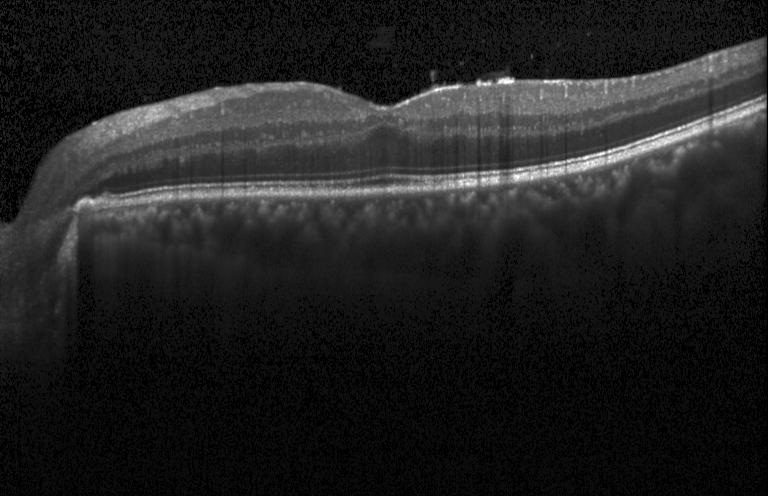 Fovea-centered, optical coherence tomography scan — No choroidal neovascularization, diabetic macular edema, or drusen.